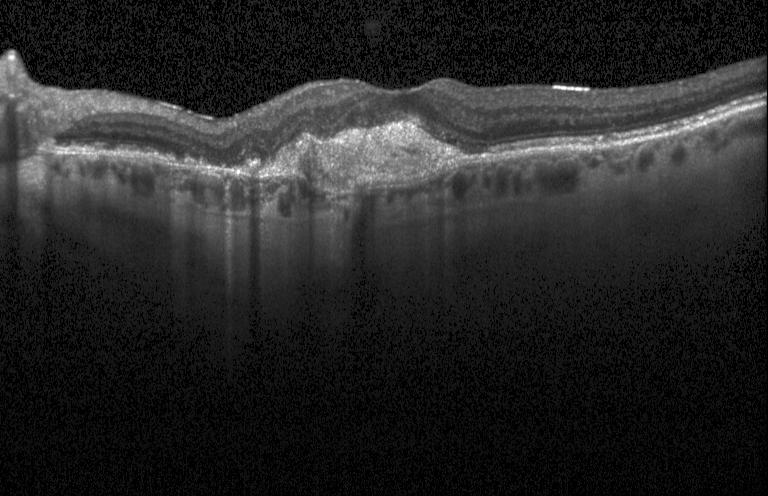 Retinal OCT B-scan — Finding: choroidal neovascularization (CNV).